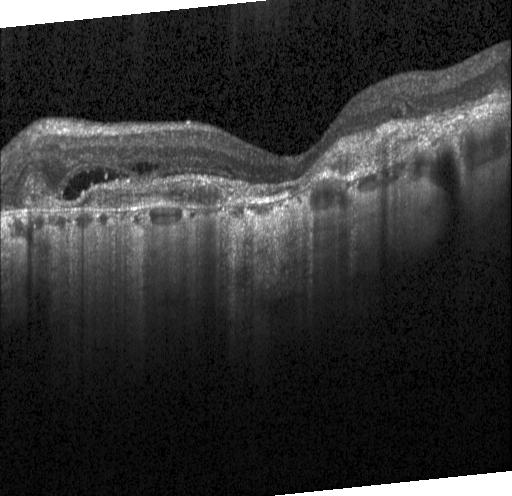 OCT B-scan showing choroidal neovascularization (CNV).